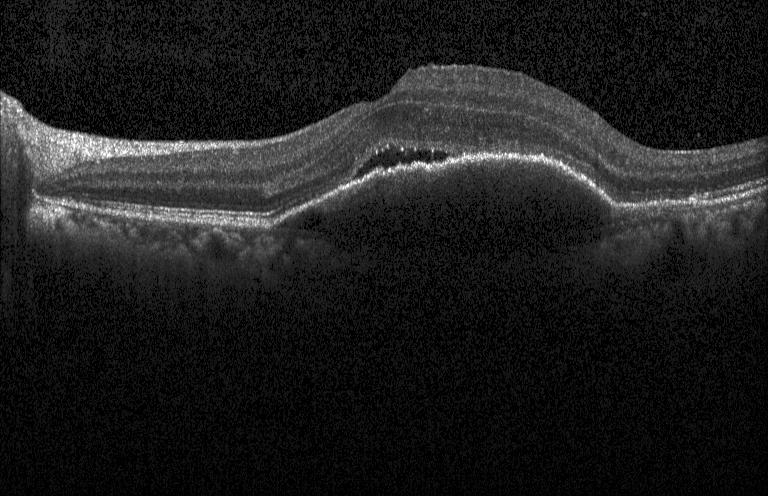 Diagnosis: choroidal neovascularization (CNV).